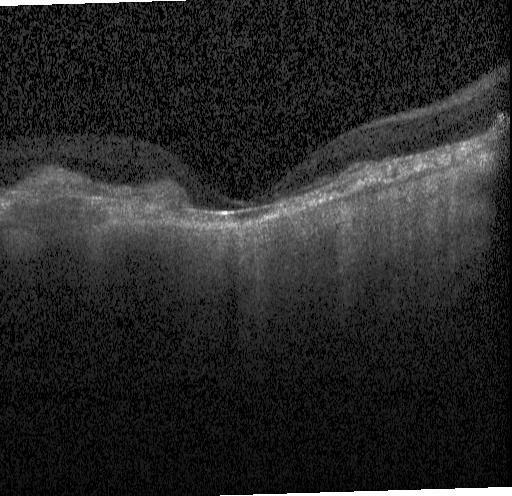
Retinal OCT cross-section showing choroidal neovascularization (CNV).